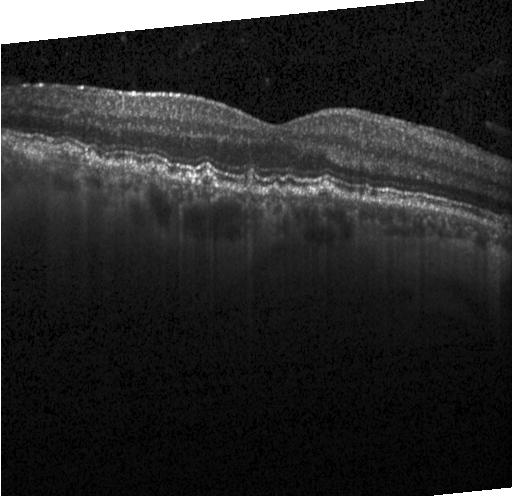

Macular scan. Spectral-domain OCT. Heidelberg Spectralis OCT system. Retinal OCT cross-section
Macular OCT: sub-RPE drusenoid deposits.